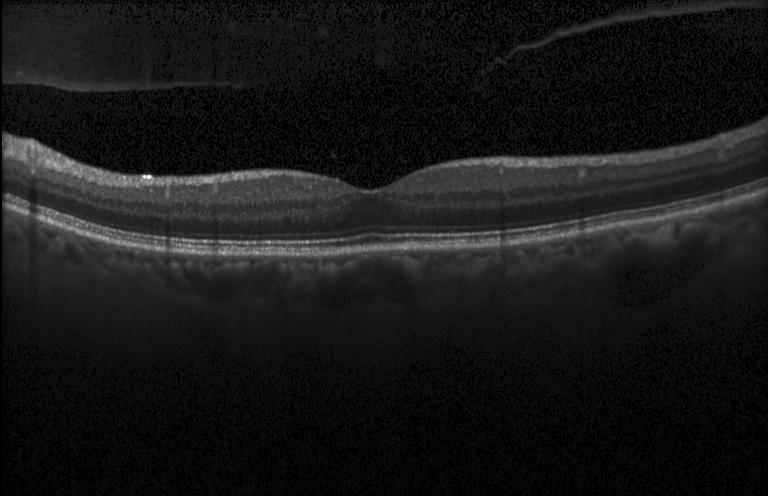 This B-scan demonstrates neither choroidal neovascularization, diabetic macular edema, nor drusen.